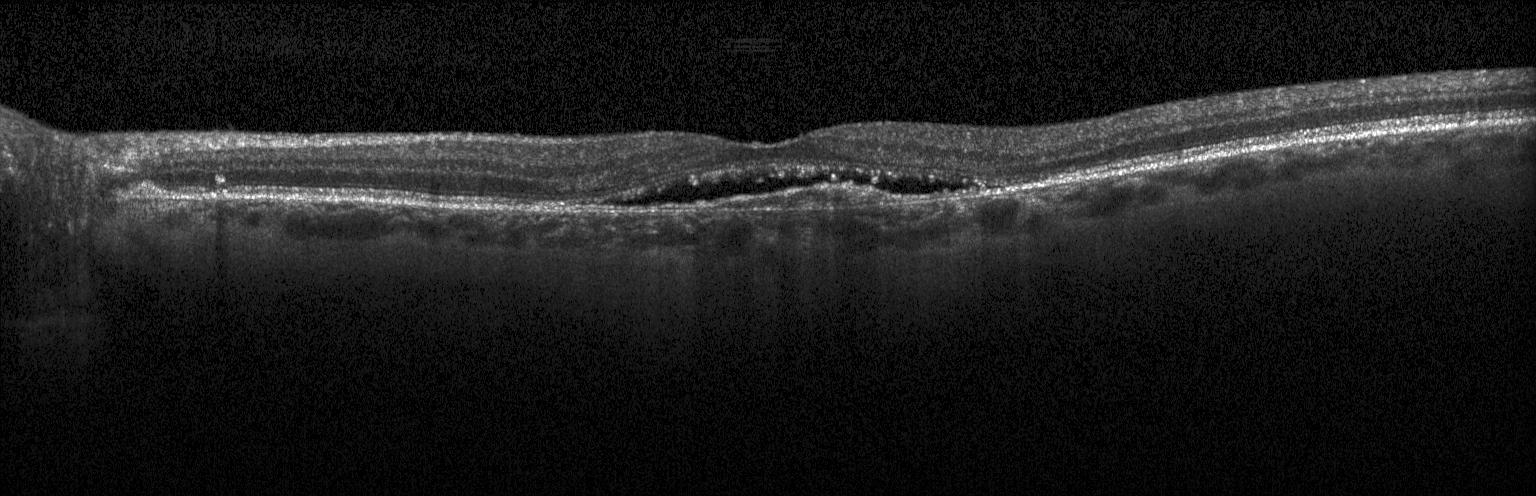

Diagnosis: a choroidal neovascular membrane.